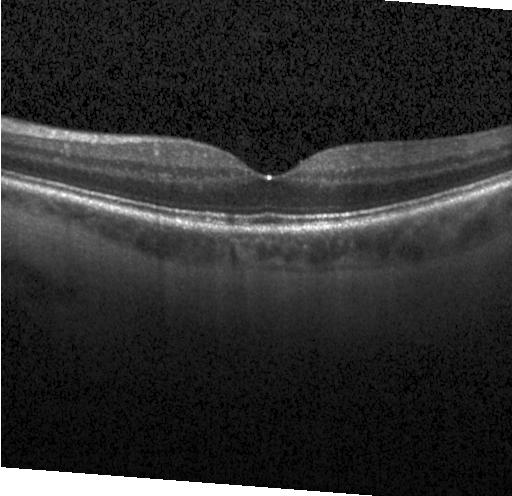 Impression: no CNV, DME, or drusen.